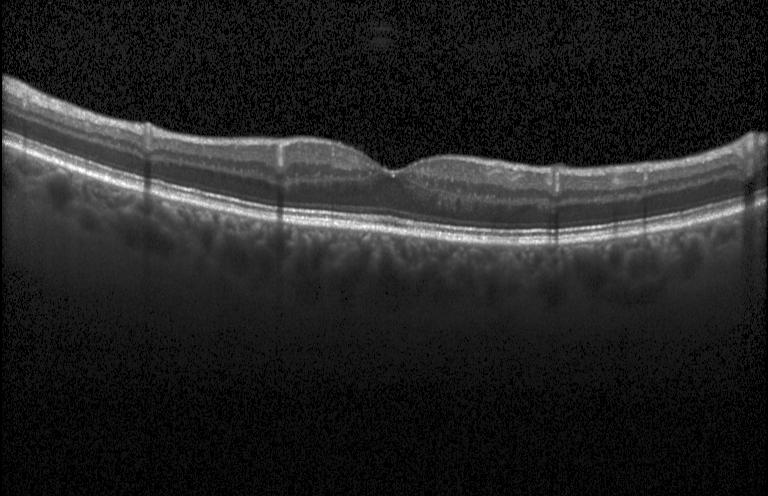
Finding: no CNV, DME, or drusen.